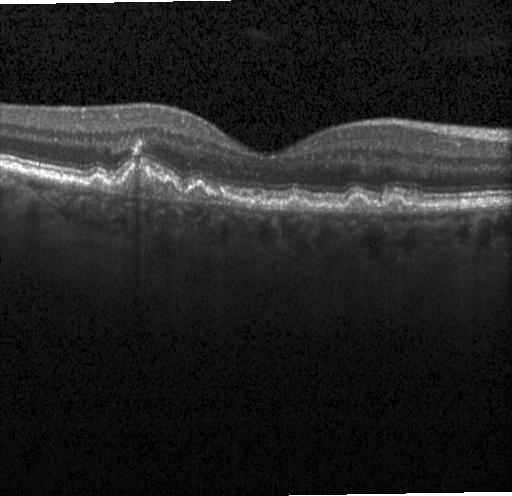 Optical coherence tomography B-scan. OCT finding: choroidal neovascularization.